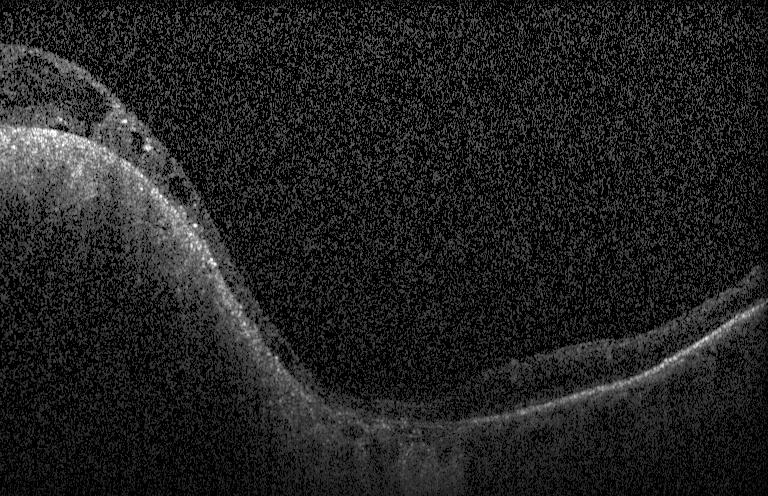

Spectral-domain optical coherence tomography. Heidelberg Spectralis OCT system. OCT line scan. Centered on the fovea — Diagnosis: diabetic macular edema (DME).